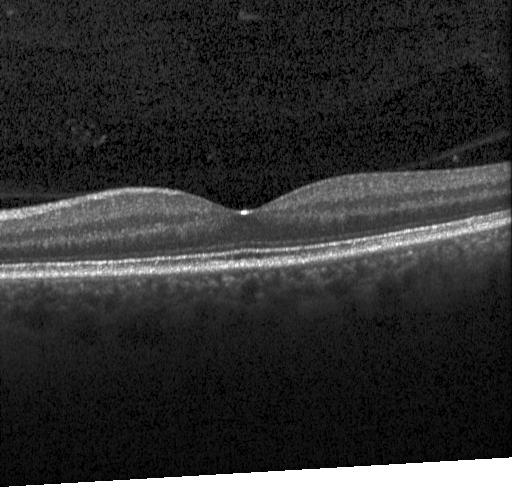

Macular OCT: no choroidal neovascularization, no diabetic macular edema, and no drusen.